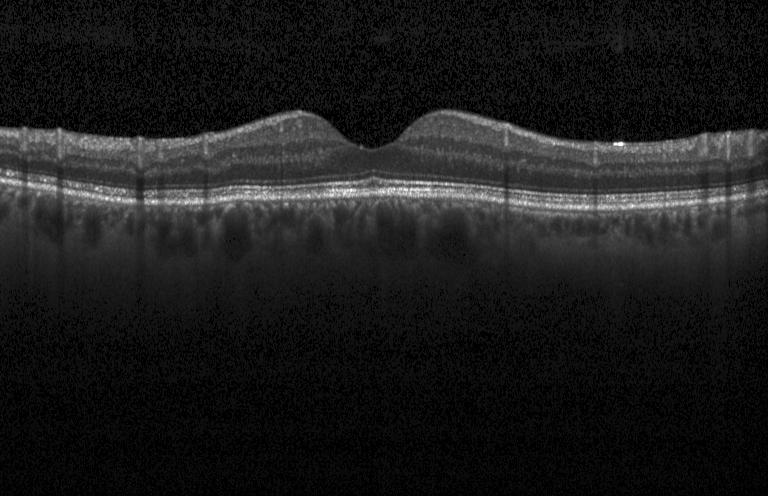
OCT line scan. Fovea-centered — No CNV, DME, or drusen.